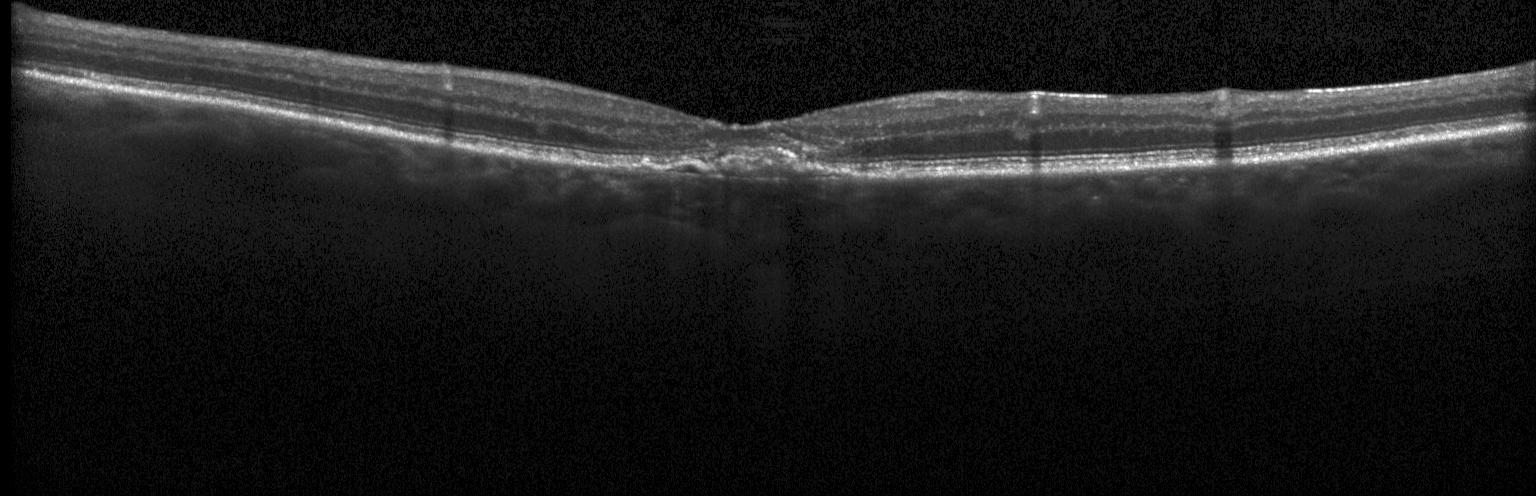

Optical coherence tomography B-scan. Heidelberg Spectralis OCT system. Through the macula. Spectral-domain optical coherence tomography — Dx: a choroidal neovascular membrane.